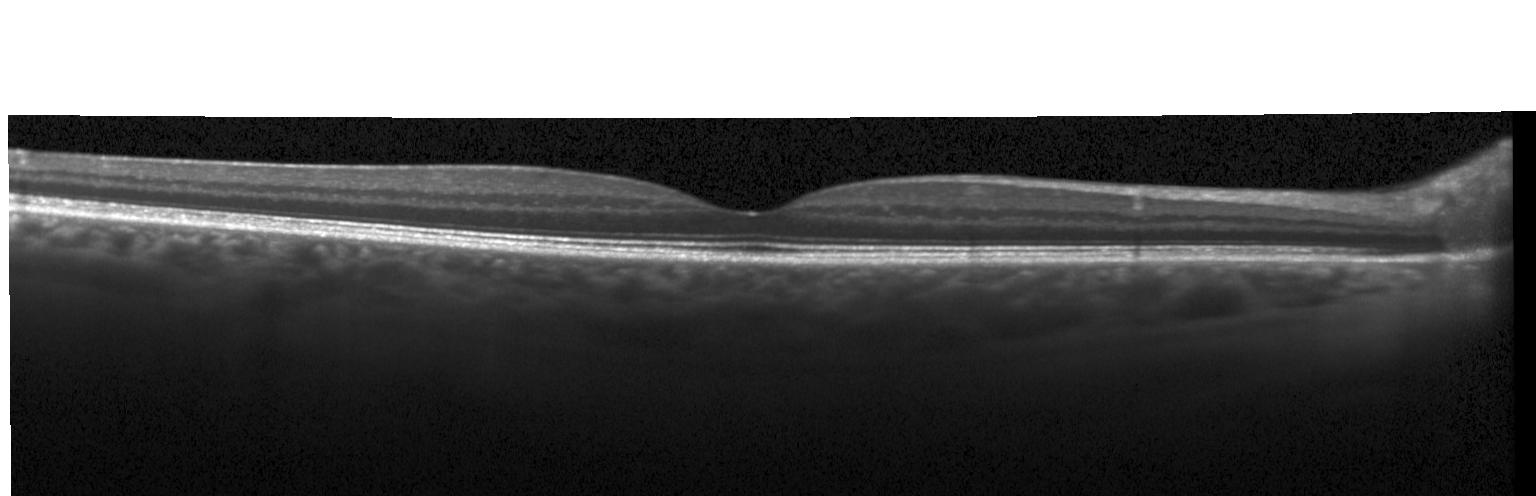

Optical coherence tomography scan. Spectral-domain optical coherence tomography. Through the macula. Acquired on a Heidelberg Spectralis.
Impression: no CNV, no DME, and no drusen.